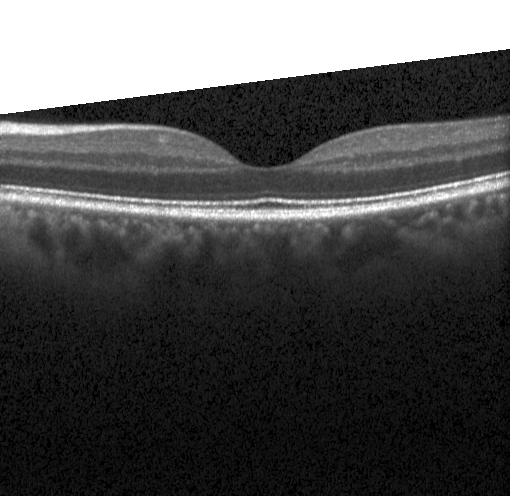

Macular OCT: no choroidal neovascularization, no diabetic macular edema, and no drusen.